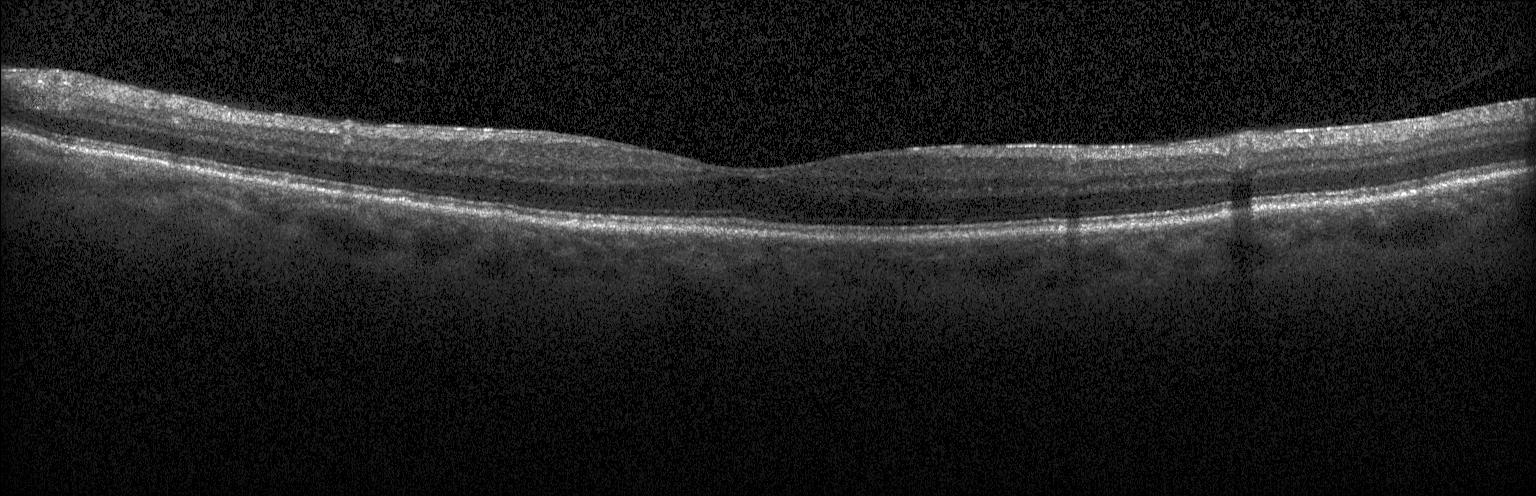
OCT B-scan — Dx: no evidence of choroidal neovascularization, diabetic macular edema, or drusen.